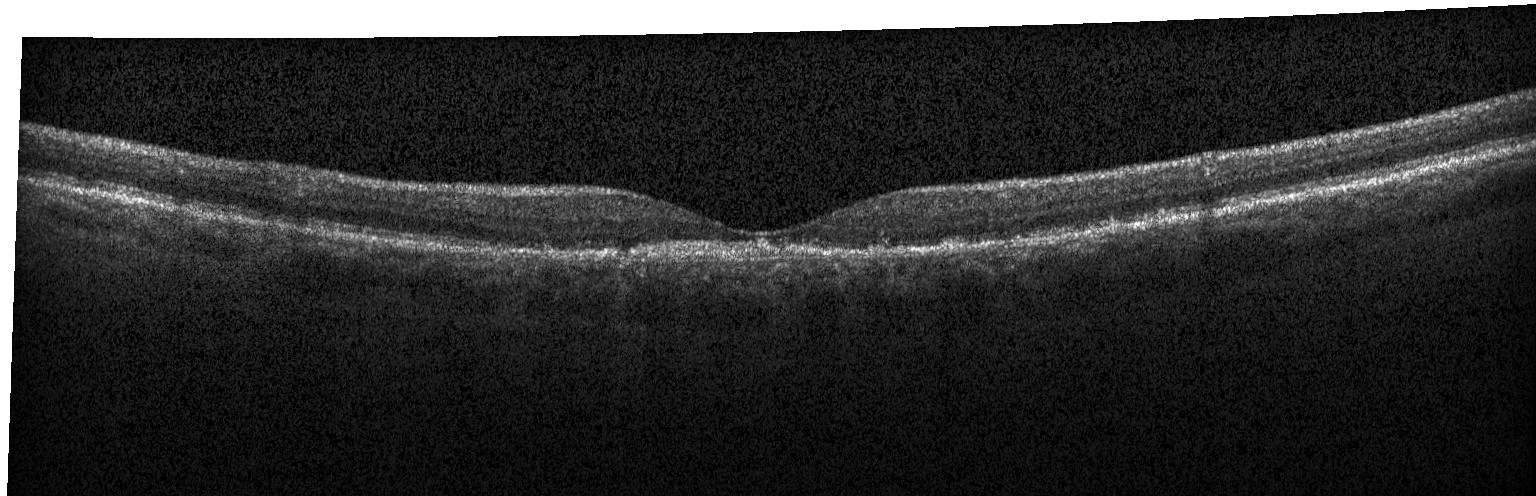
Dx: CNV.